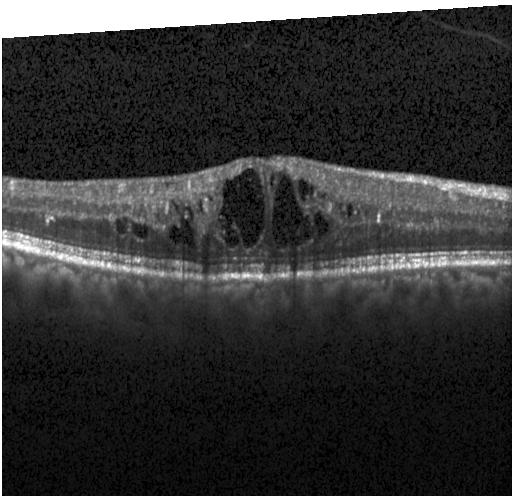

Dx: diabetic macular edema (DME).